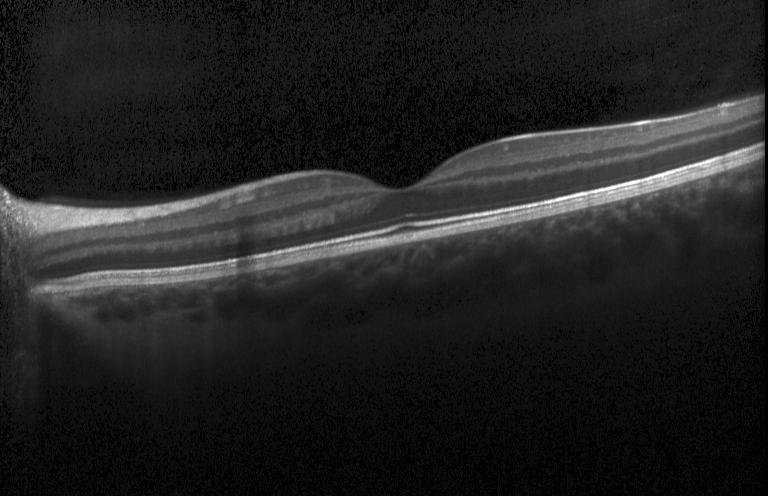
OCT line scan, centered on the fovea, Heidelberg Spectralis, SD-OCT
Finding: no choroidal neovascularization, no diabetic macular edema, and no drusen.